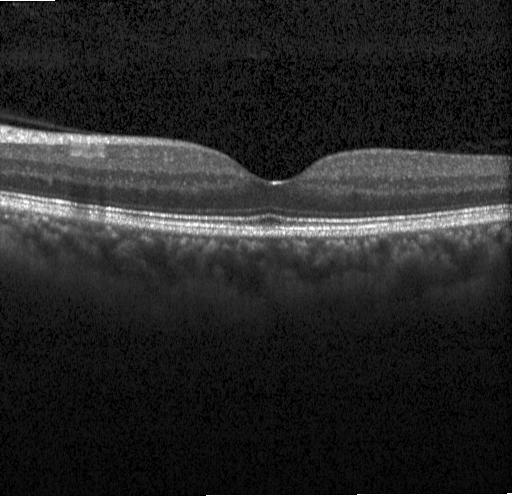

Heidelberg Spectralis OCT system · OCT B-scan — Diagnosis: no choroidal neovascularization, diabetic macular edema, or drusen.